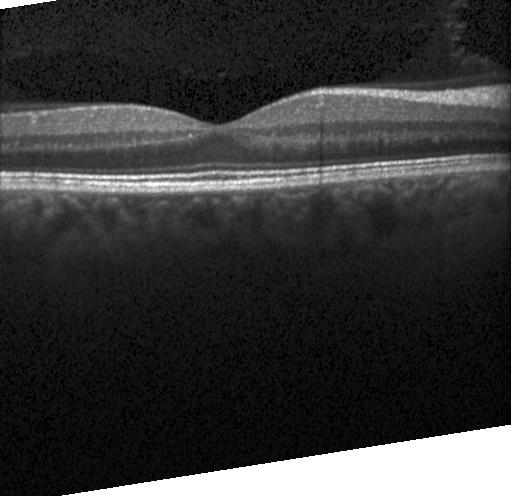 Macular OCT demonstrating no choroidal neovascularization, diabetic macular edema, or drusen.